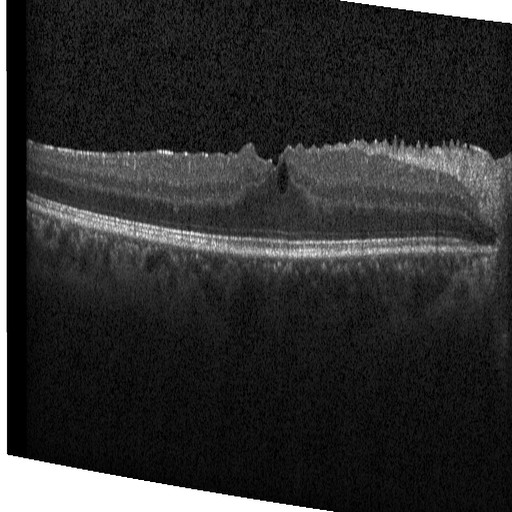

Diagnosis: diabetic macular edema (DME).